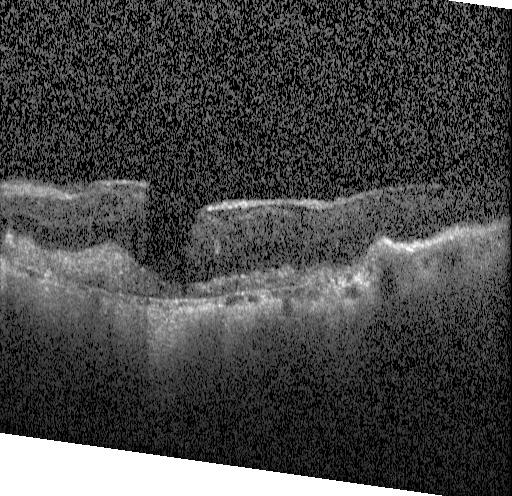 Choroidal neovascularization.